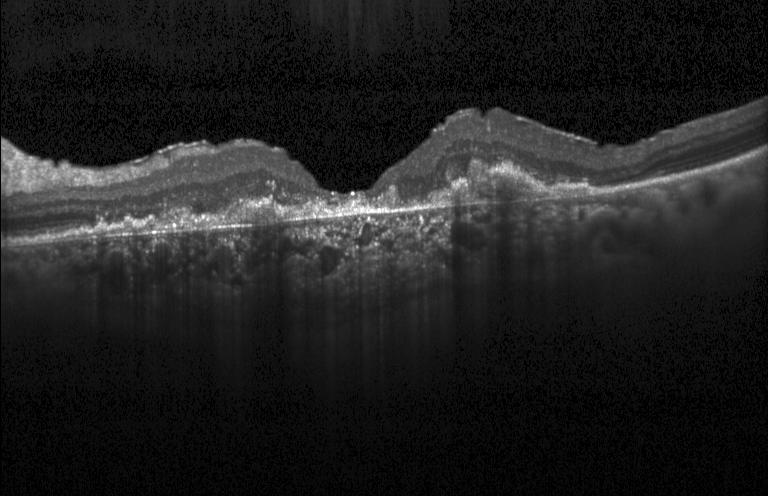

Spectral-domain OCT, through the macula, optical coherence tomography B-scan, instrument: Heidelberg Spectralis — This B-scan demonstrates choroidal neovascularization.